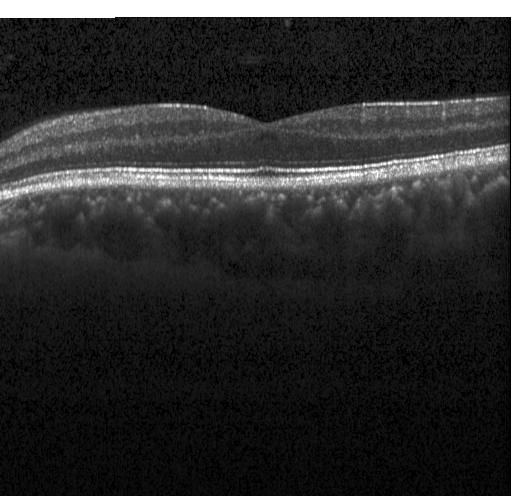

Optical coherence tomography scan, centered on the fovea, instrument: Heidelberg Spectralis, SD-OCT
Diagnosis: neither choroidal neovascularization, diabetic macular edema, nor drusen.